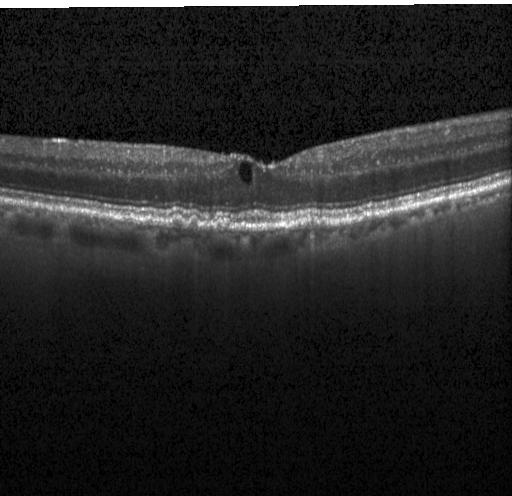

Retinal OCT cross-section — Diagnosis: DME.